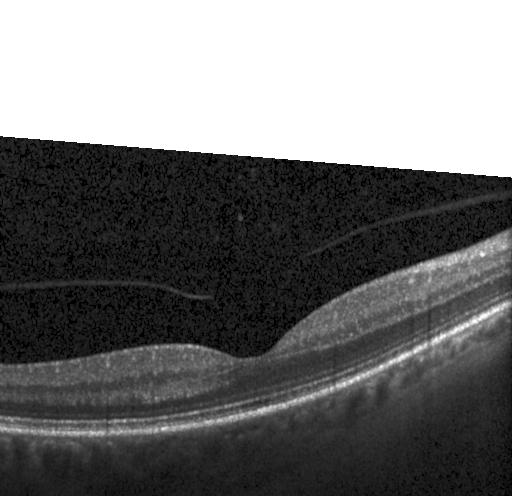 OCT scan showing no CNV, no DME, and no drusen.